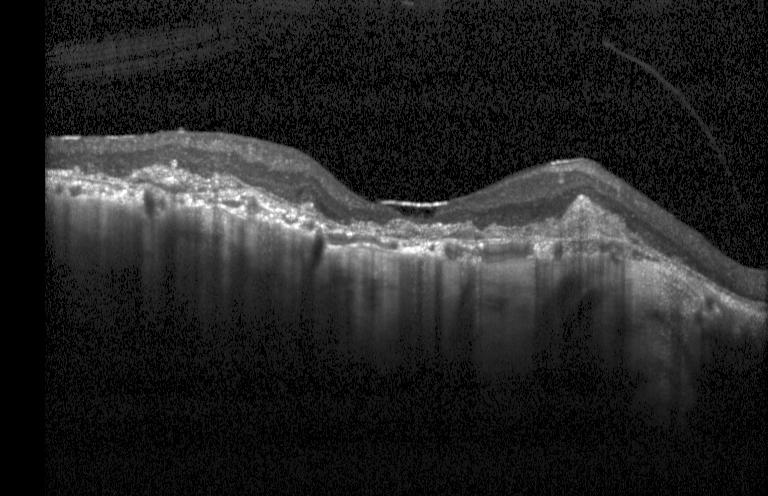

Assessment: choroidal neovascularization.